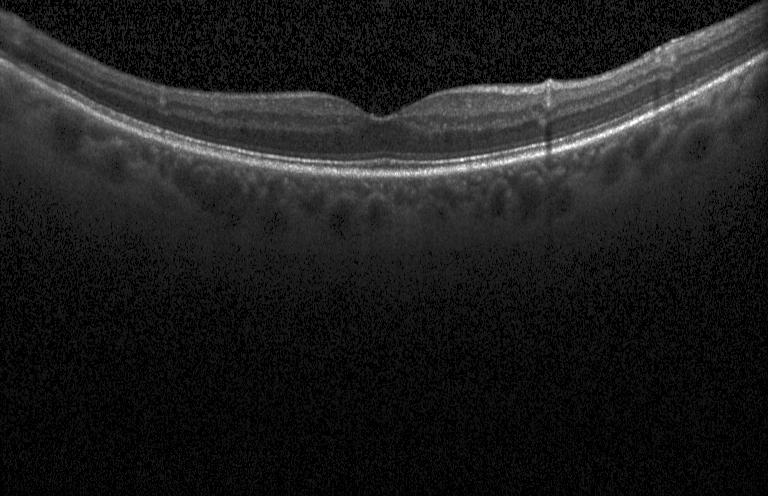

Instrument: Heidelberg Spectralis, SD-OCT, horizontal scan through the fovea, optical coherence tomography scan — Impression: neither choroidal neovascularization, diabetic macular edema, nor drusen.